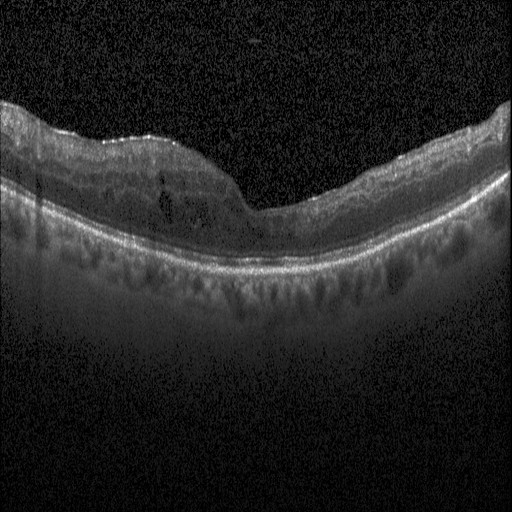
Acquired on a Heidelberg Spectralis · optical coherence tomography B-scan · horizontal scan through the fovea · spectral-domain optical coherence tomography — Finding: DME.